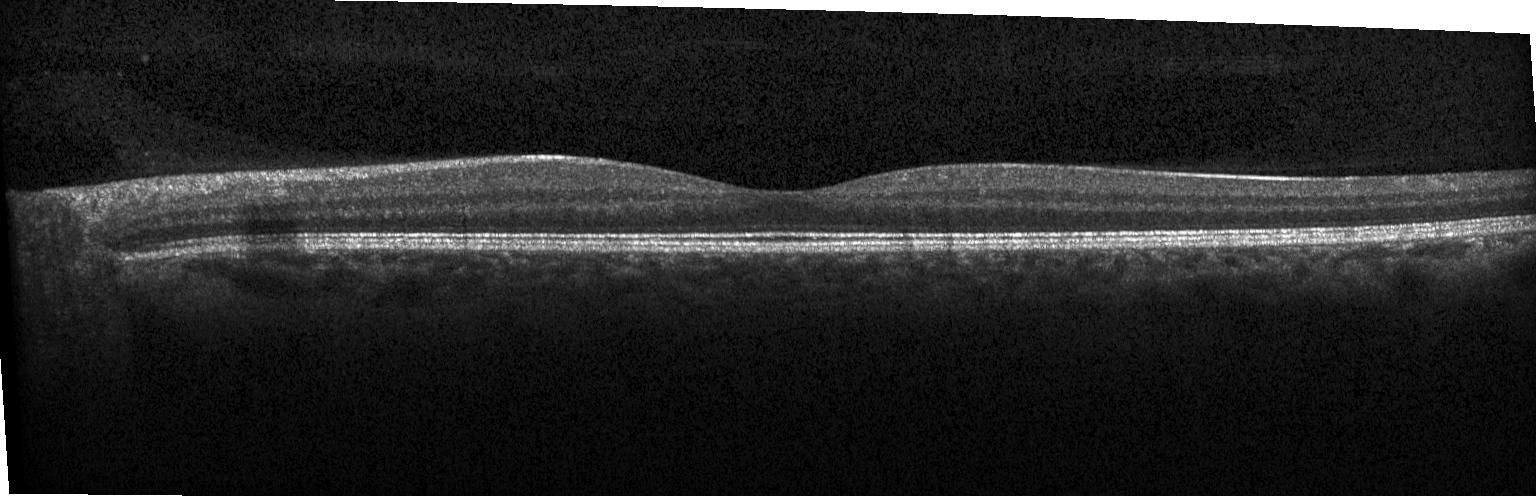

OCT line scan
The scan shows neither choroidal neovascularization, diabetic macular edema, nor drusen.